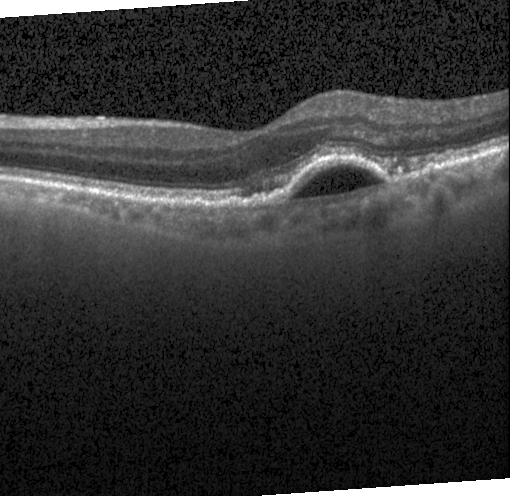
The scan shows a choroidal neovascular membrane.